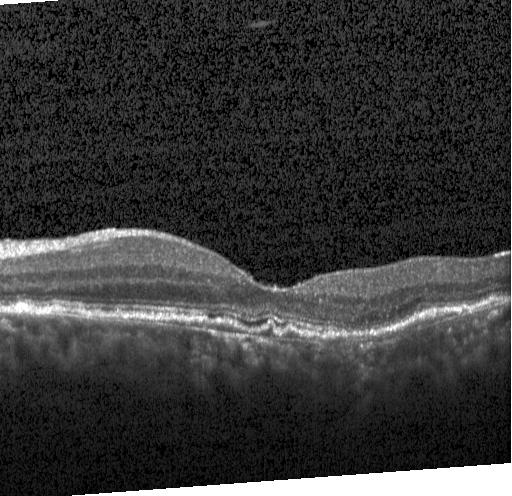 Spectral-domain OCT B-scan: a choroidal neovascular membrane.